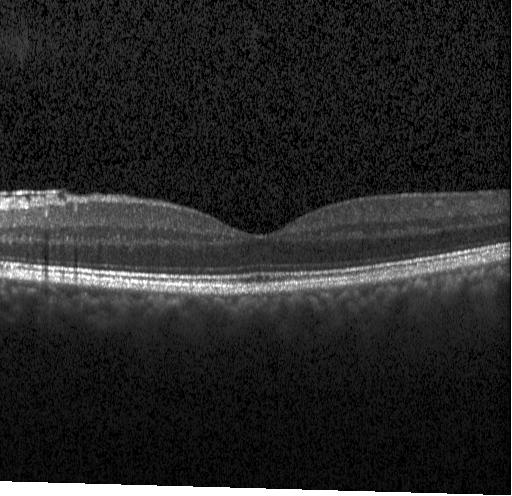
This B-scan demonstrates neither choroidal neovascularization, diabetic macular edema, nor drusen.